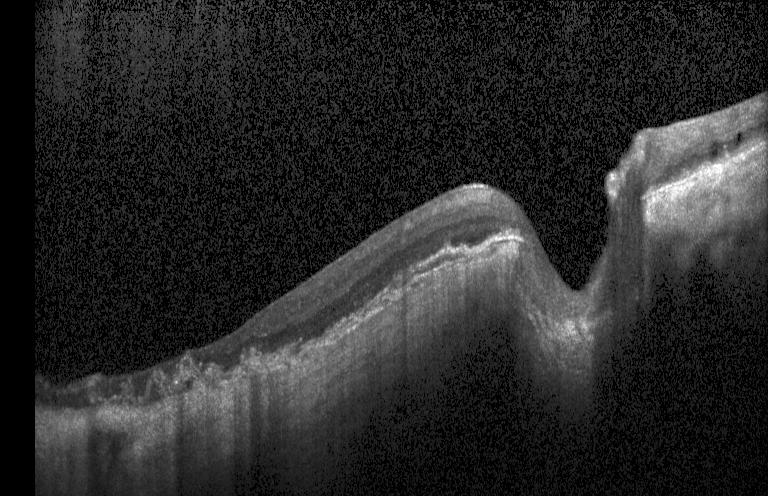
Impression: choroidal neovascularization.